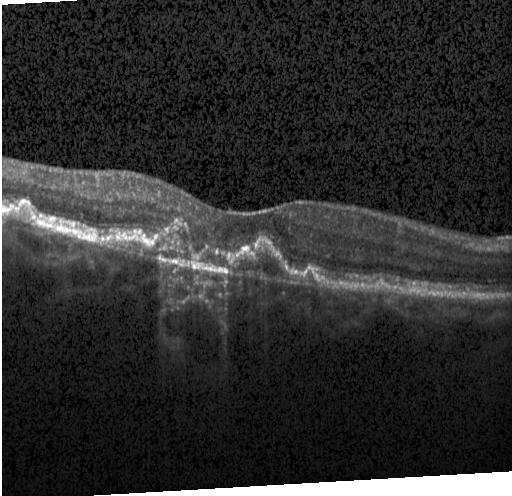
SD-OCT. Instrument: Heidelberg Spectralis. Macular scan. Retinal OCT cross-section.
Impression: CNV.